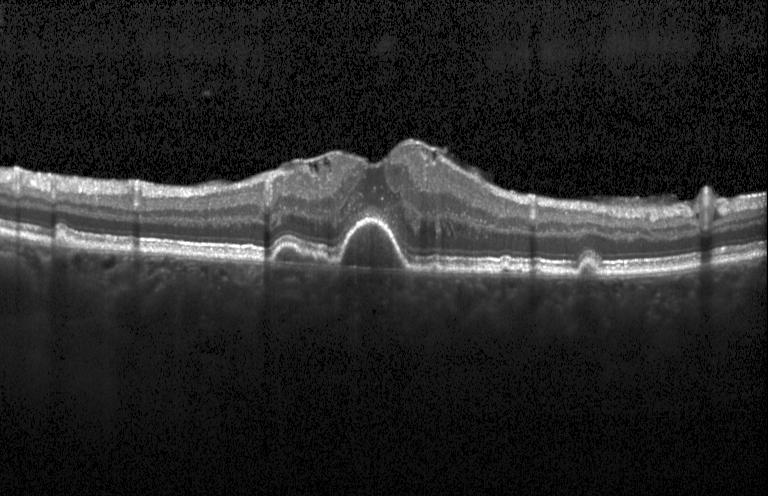 Dx: a choroidal neovascular membrane.